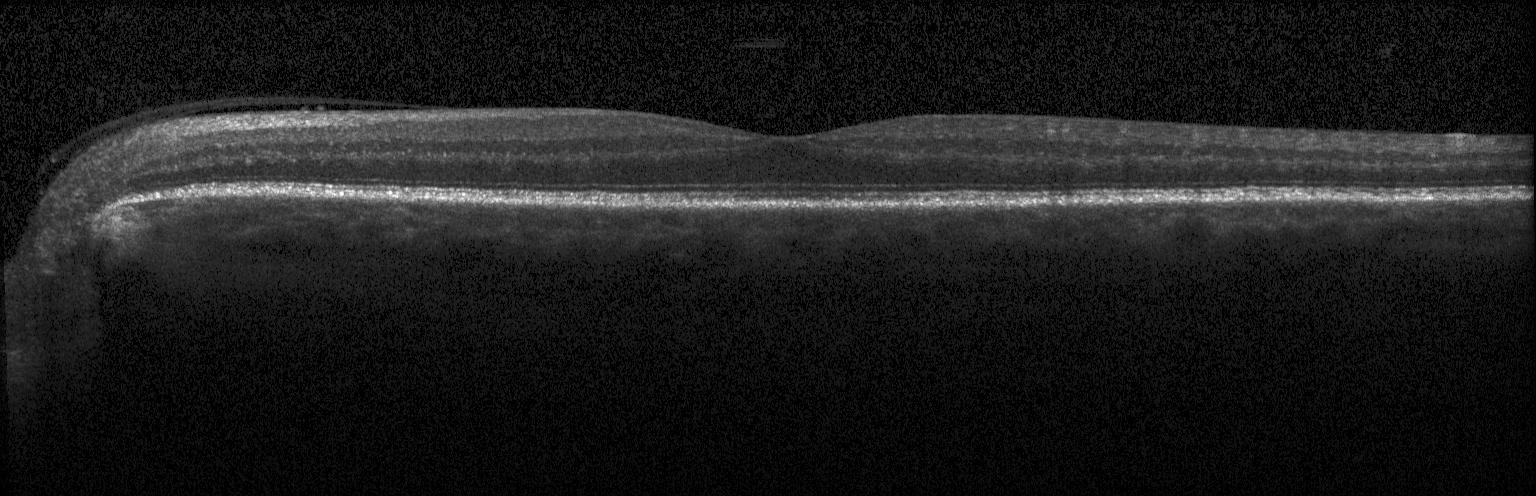
Spectral-domain OCT, Heidelberg Spectralis OCT system, OCT B-scan, fovea-centered.
Finding: neither choroidal neovascularization, diabetic macular edema, nor drusen.